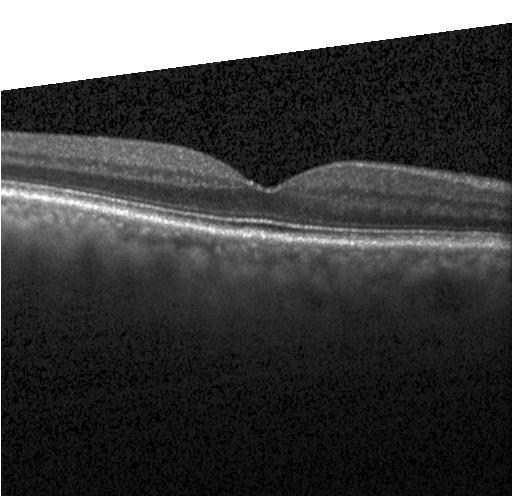

Heidelberg Spectralis OCT system, centered on the fovea, OCT B-scan — Assessment: no choroidal neovascularization, diabetic macular edema, or drusen.